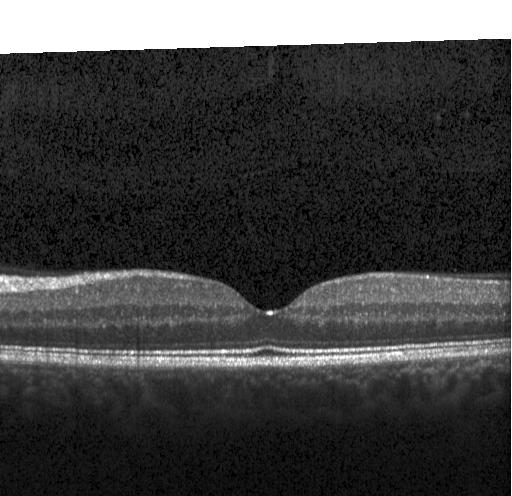 OCT scan showing neither choroidal neovascularization, diabetic macular edema, nor drusen.